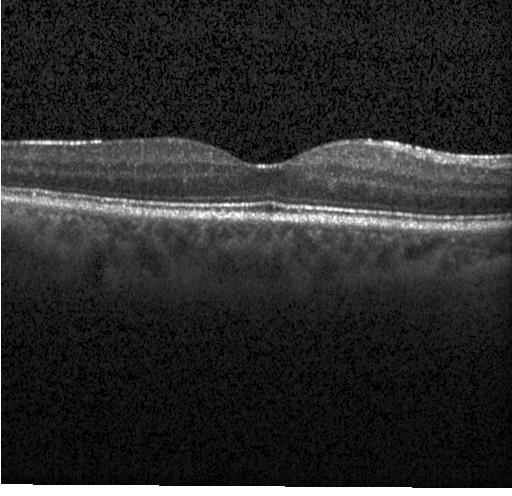 Through the macula, SD-OCT, Heidelberg Spectralis, retinal OCT cross-section
Finding: neither choroidal neovascularization, diabetic macular edema, nor drusen.